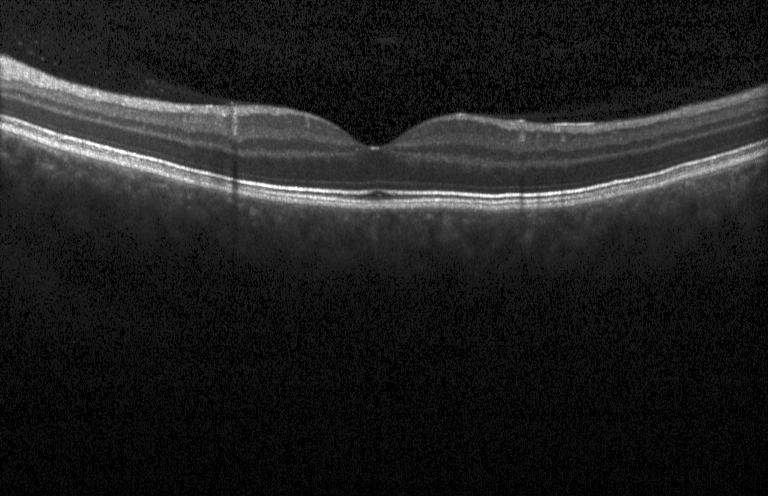 Assessment: neither choroidal neovascularization, diabetic macular edema, nor drusen.